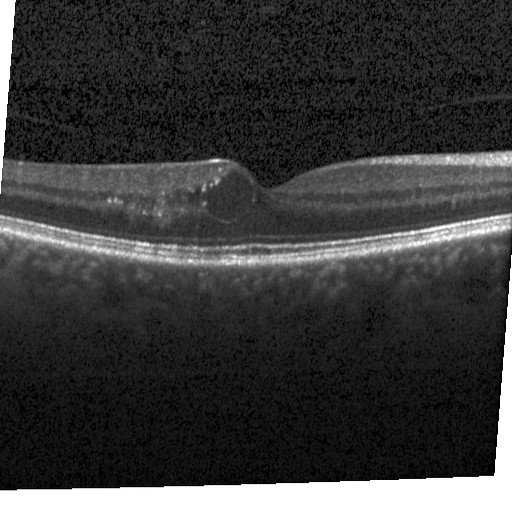 Diabetic macular edema (DME).